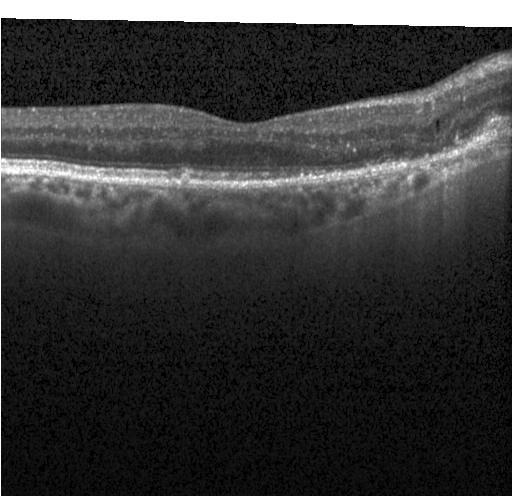
Spectral-domain OCT B-scan: a choroidal neovascular membrane.